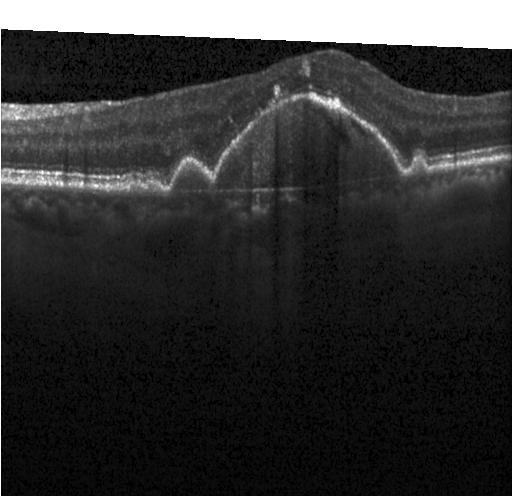

OCT scan showing CNV.